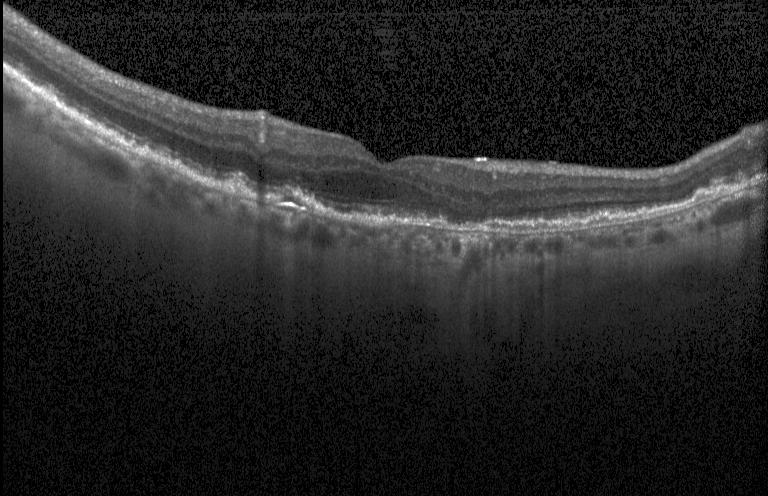
OCT scan showing a choroidal neovascular membrane.